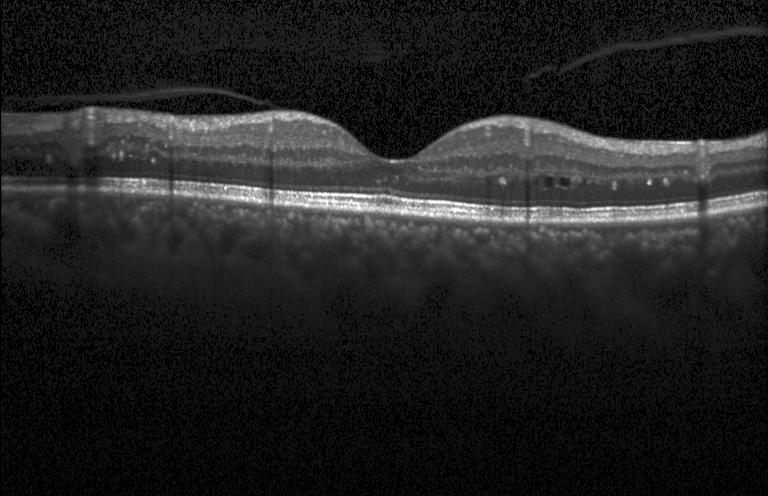
Through the macula; acquired on a Heidelberg Spectralis; retinal OCT cross-section; spectral-domain optical coherence tomography — Diagnosis: diabetic macular edema.